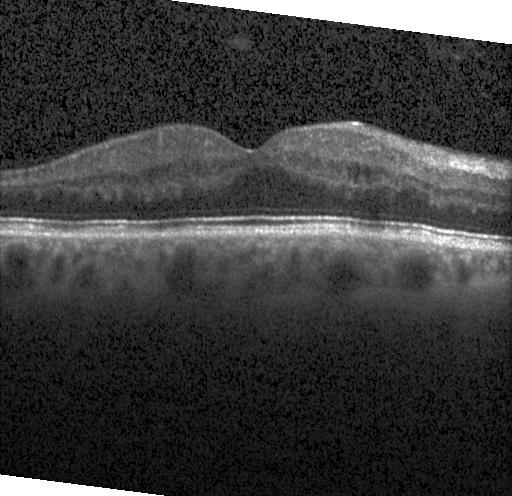 Optical coherence tomography scan, fovea-centered, Heidelberg Spectralis OCT system — OCT finding: DME.